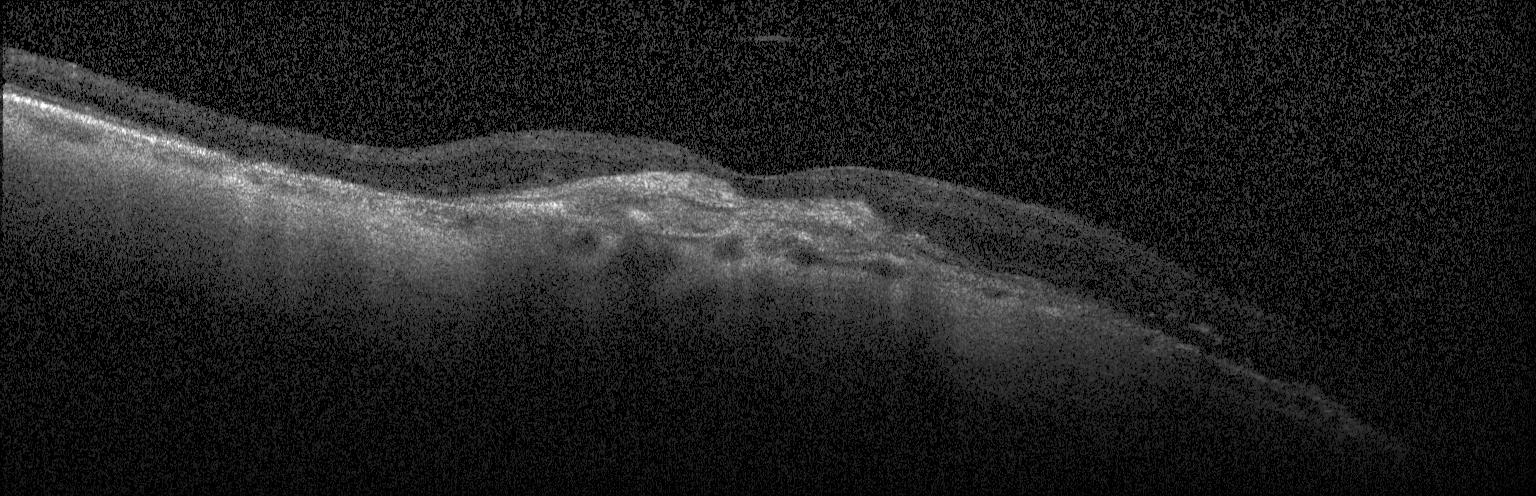 Diagnosis: a choroidal neovascular membrane.